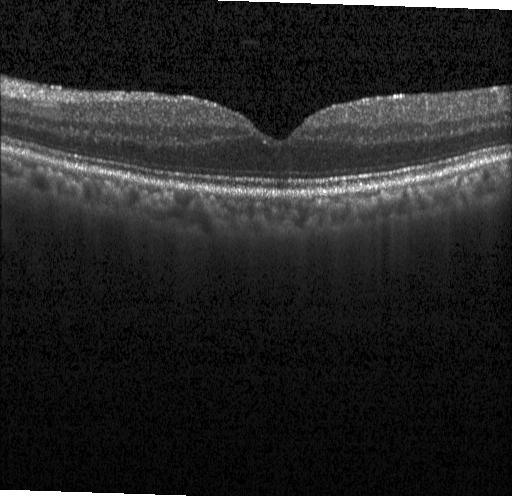 Retinal OCT cross-section — Impression: no CNV, no DME, and no drusen.